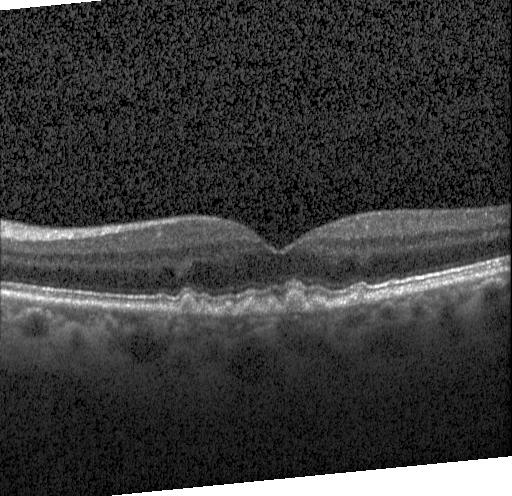

Optical coherence tomography scan. Spectral-domain OCT.
Diagnosis: drusen.